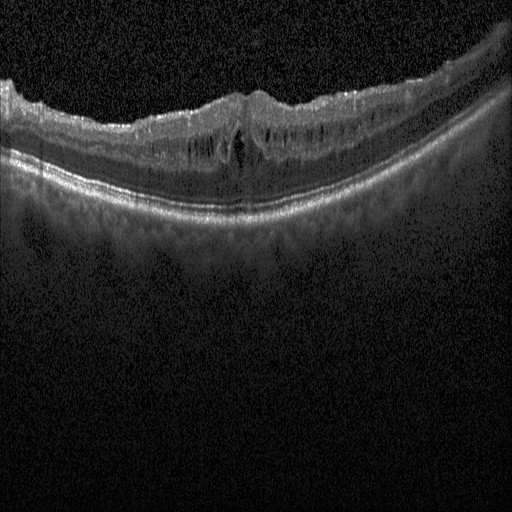

SD-OCT, centered on the fovea, OCT B-scan, Heidelberg Spectralis OCT system — Finding: diabetic macular edema.